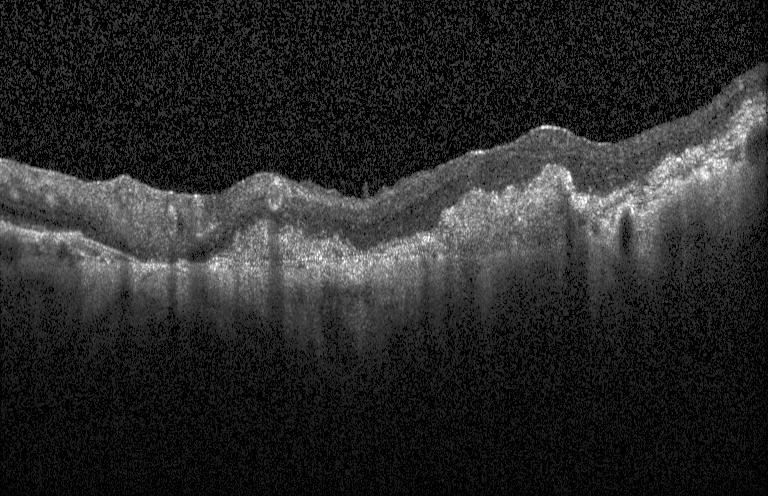
OCT line scan. Spectral-domain optical coherence tomography. Centered on the fovea. Heidelberg Spectralis OCT system — The scan shows choroidal neovascularization (CNV).